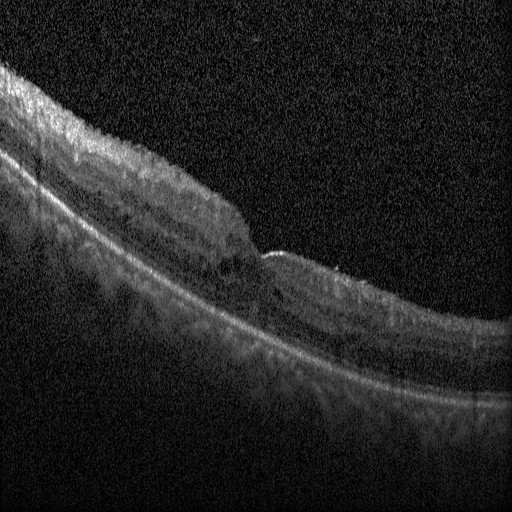

Horizontal scan through the fovea. Optical coherence tomography B-scan
Finding: DME.